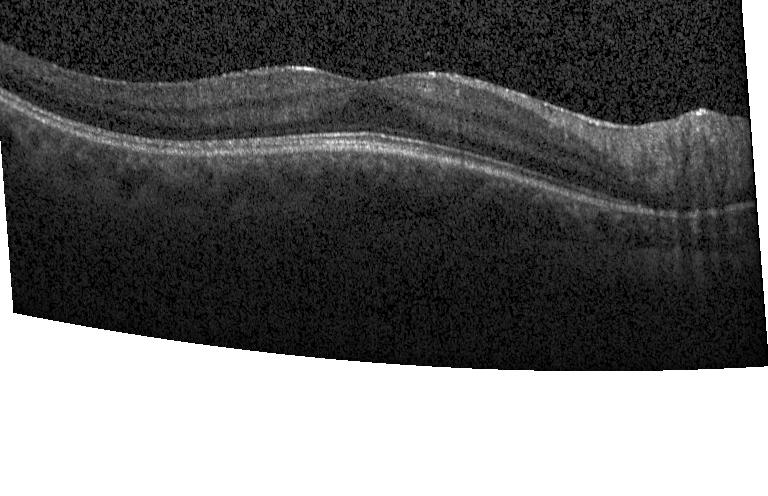

OCT B-scan, instrument: Heidelberg Spectralis — The scan shows no evidence of choroidal neovascularization, diabetic macular edema, or drusen.